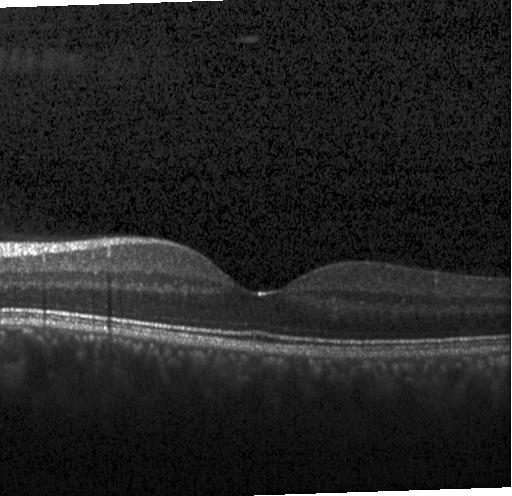 Centered on the fovea. Heidelberg Spectralis OCT system. Optical coherence tomography B-scan
Assessment: no evidence of choroidal neovascularization, diabetic macular edema, or drusen.